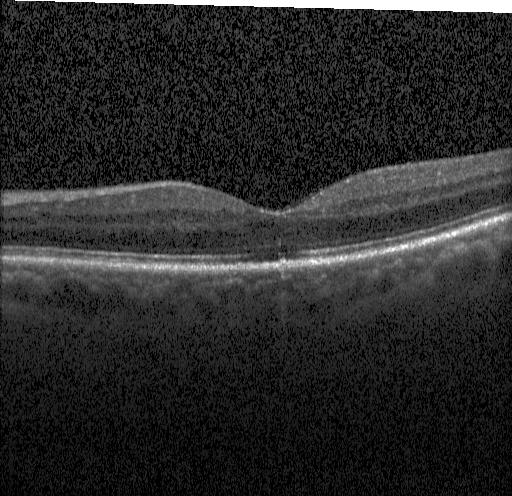

OCT B-scan; instrument: Heidelberg Spectralis; spectral-domain optical coherence tomography
OCT finding: neither CNV, DME, nor drusen.